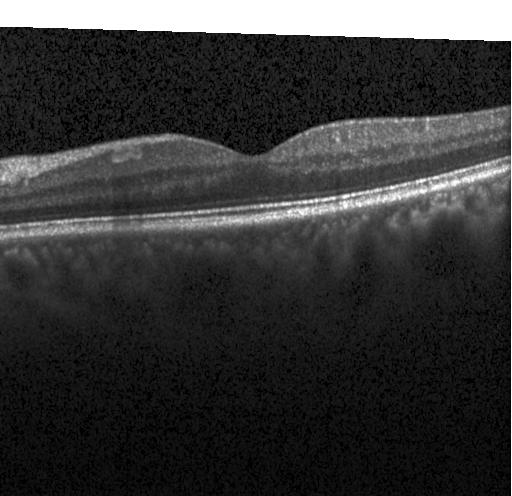
OCT B-scan showing no evidence of choroidal neovascularization, diabetic macular edema, or drusen.